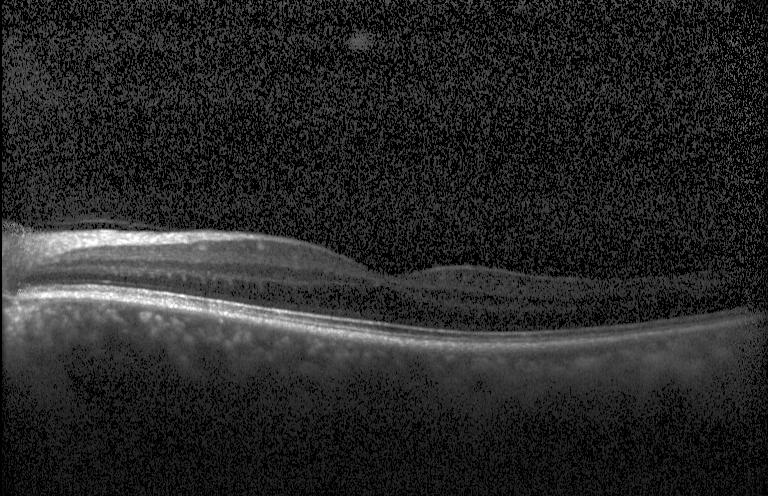
OCT finding: no choroidal neovascularization, diabetic macular edema, or drusen.